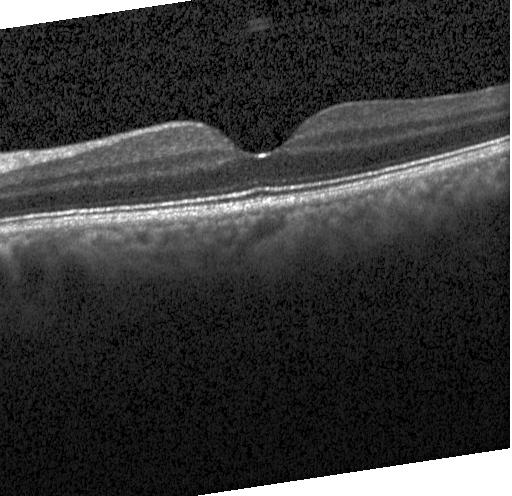
Macular OCT: no choroidal neovascularization, diabetic macular edema, or drusen.